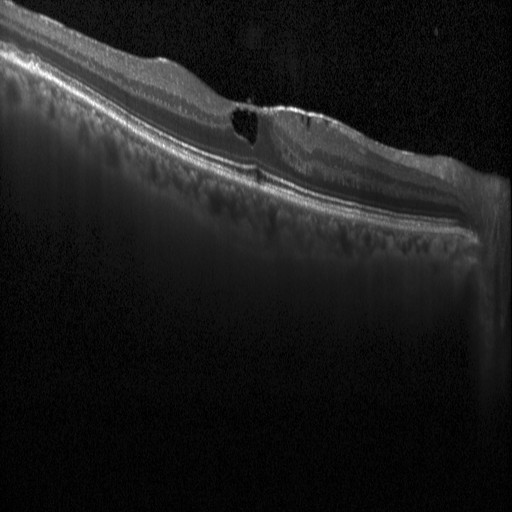

Instrument: Heidelberg Spectralis; retinal OCT cross-section; spectral-domain optical coherence tomography; macular scan
Finding: DME.